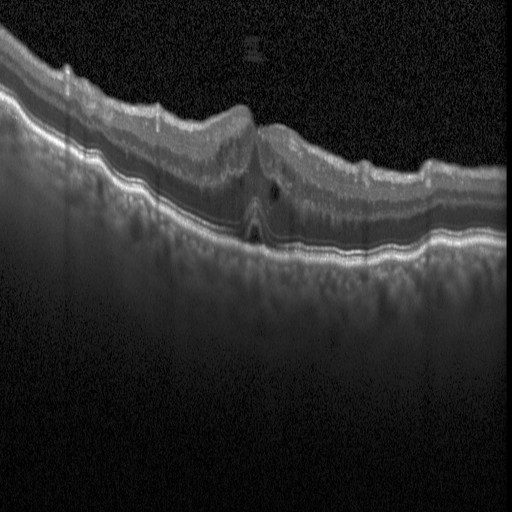 The scan shows diabetic macular edema (DME).